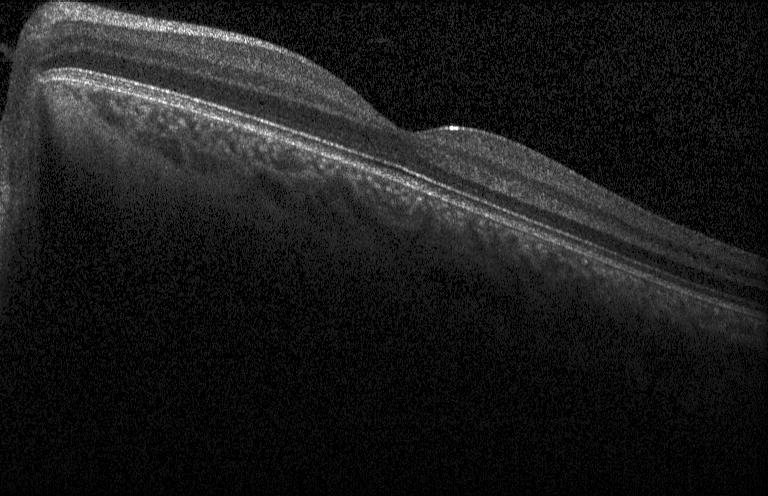 Macular OCT demonstrating no choroidal neovascularization, diabetic macular edema, or drusen.